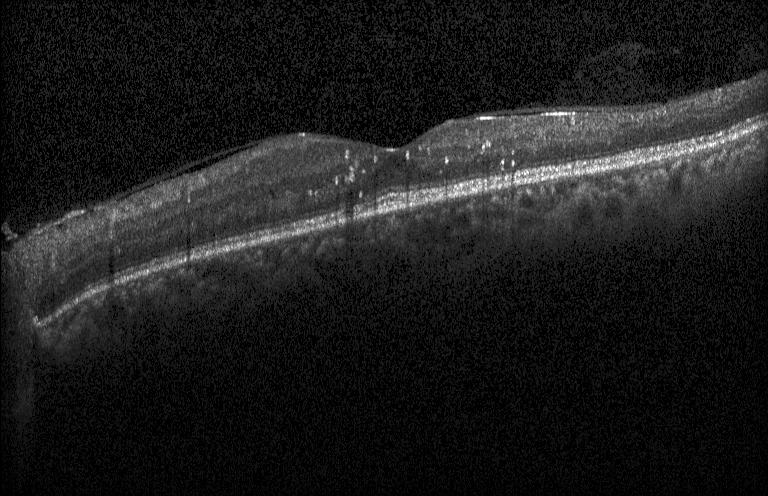 This B-scan demonstrates diabetic macular edema.